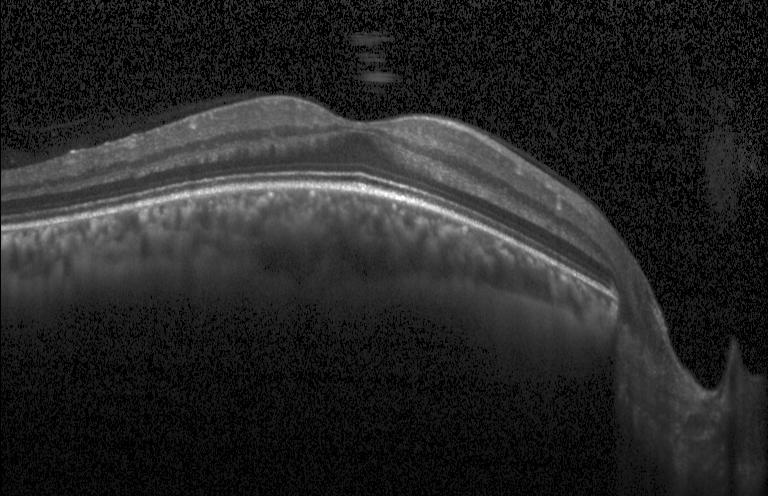

Optical coherence tomography scan; fovea-centered; Heidelberg Spectralis; spectral-domain OCT. The scan shows no choroidal neovascularization, diabetic macular edema, or drusen.